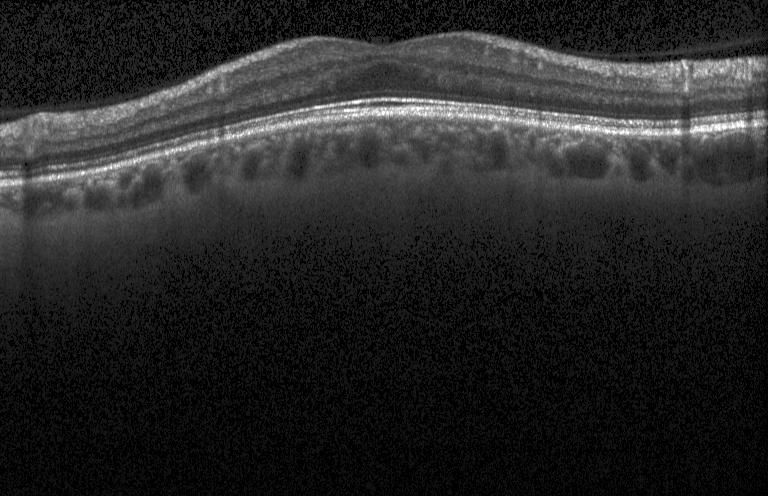

OCT line scan.
Diagnosis: no CNV, DME, or drusen.